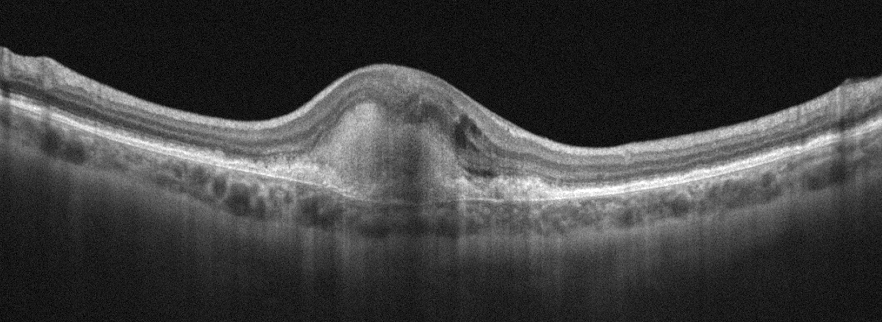

Through the macula. OCT B-scan
Impression: AMD.